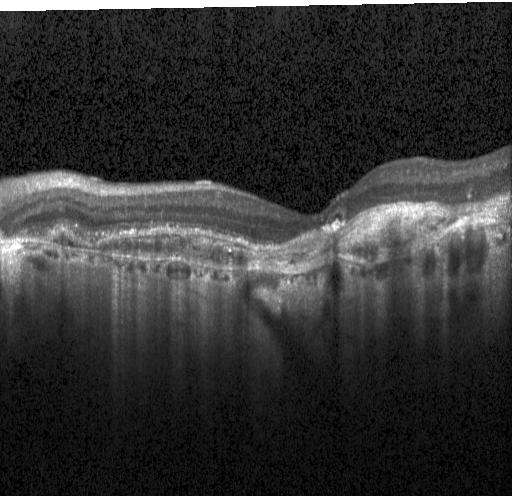
Retinal OCT cross-section showing choroidal neovascularization.